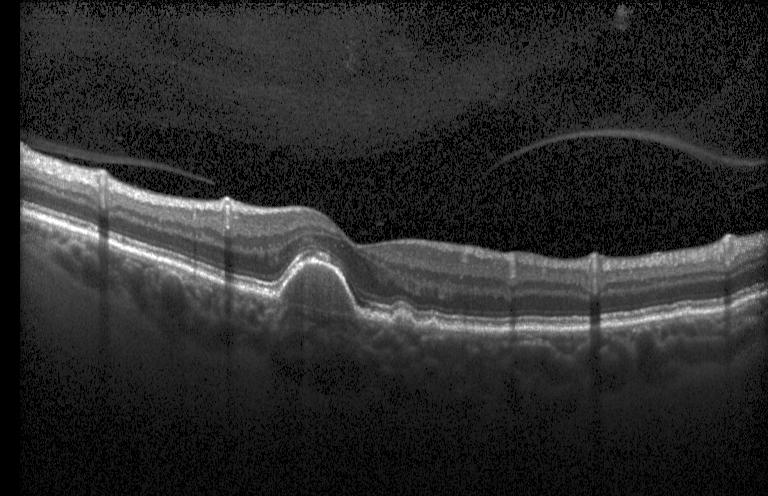

A choroidal neovascular membrane.